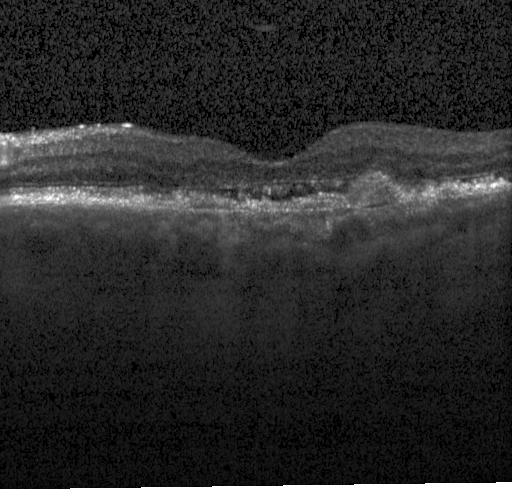 The scan shows choroidal neovascularization (CNV).